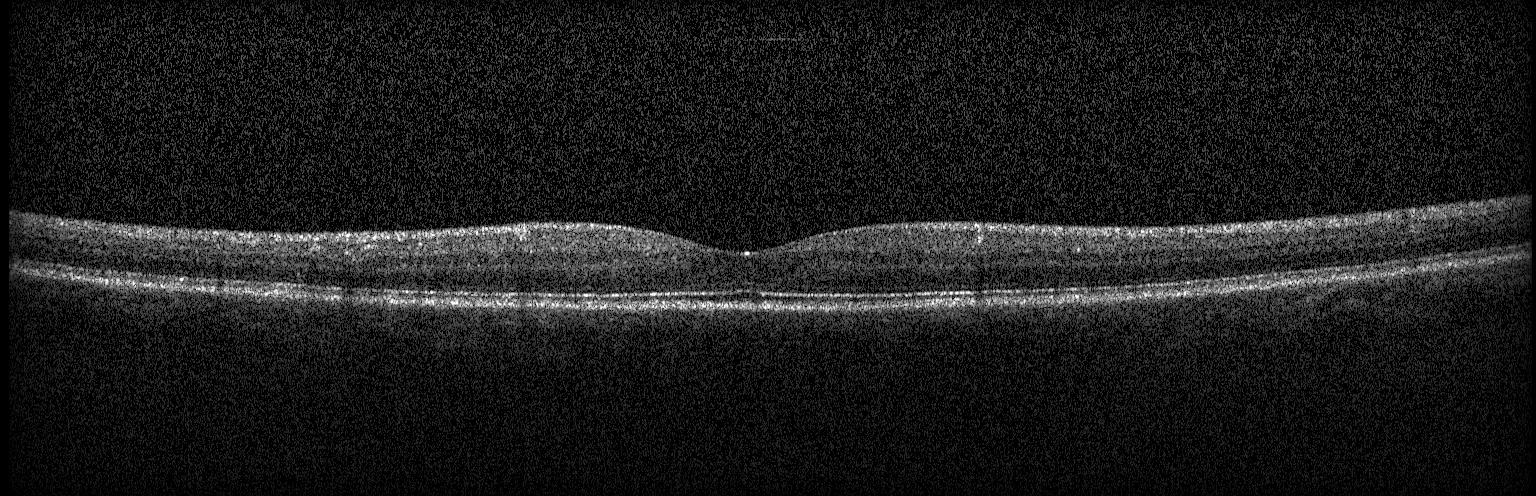

Diagnosis: no choroidal neovascularization, no diabetic macular edema, and no drusen.